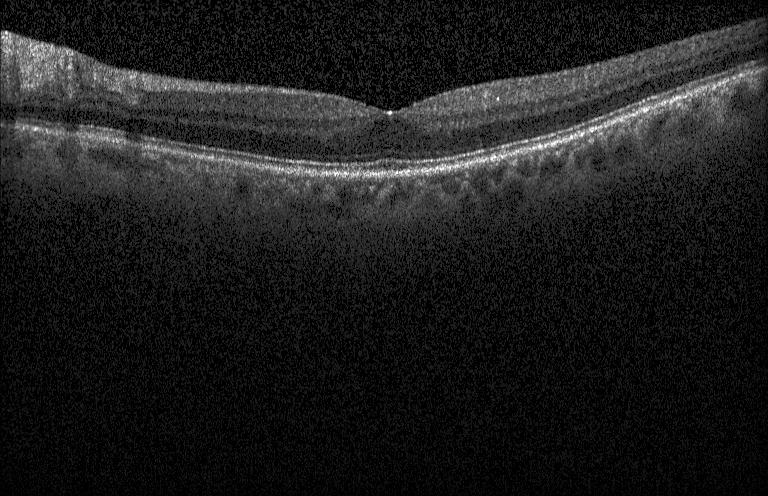 Optical coherence tomography B-scan
Impression: no evidence of CNV, DME, or drusen.